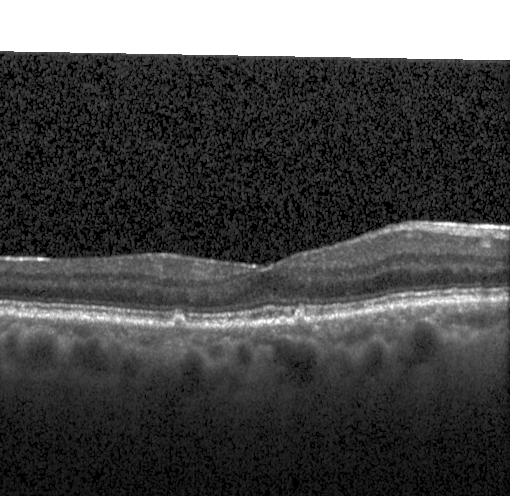 Retinal OCT cross-section showing drusen.